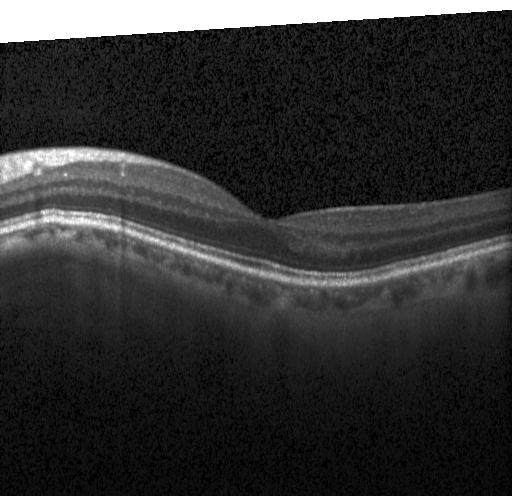 Macular OCT: no choroidal neovascularization, no diabetic macular edema, and no drusen.